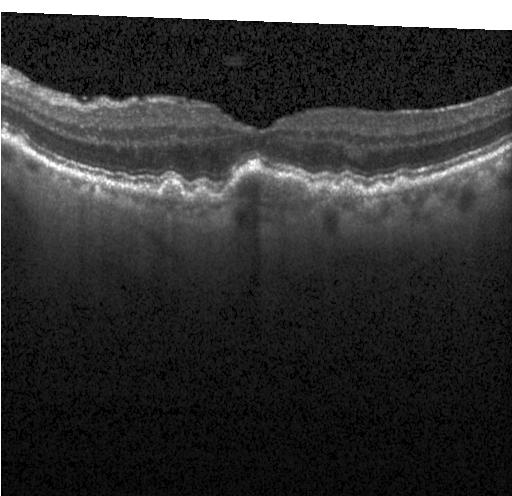
Finding: CNV.